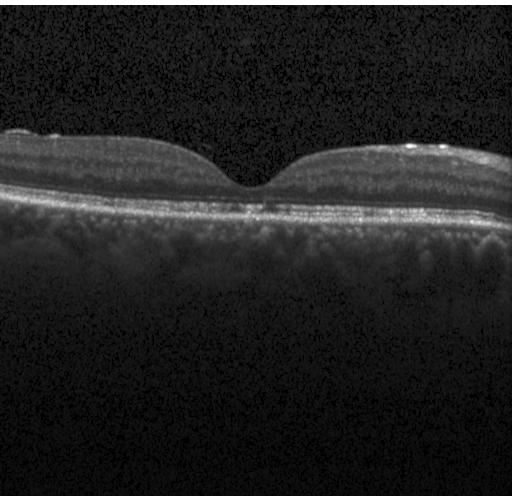

Diagnosis: neither choroidal neovascularization, diabetic macular edema, nor drusen.